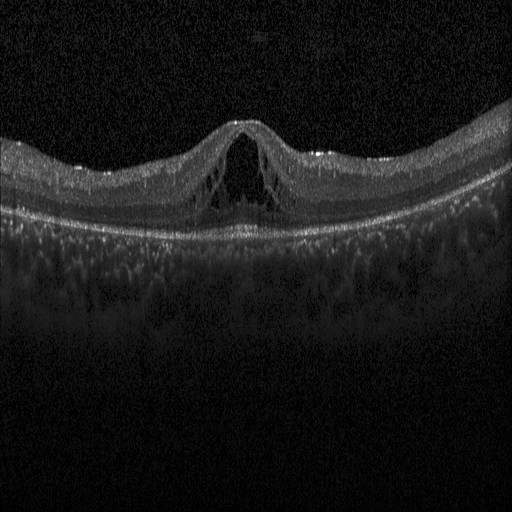

OCT finding: diabetic macular edema.